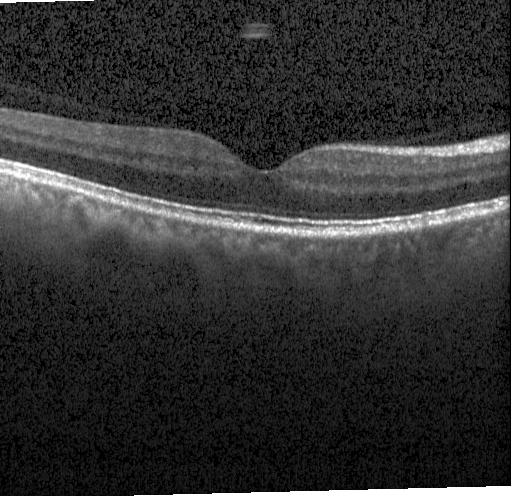 Optical coherence tomography scan. Diagnosis: no evidence of choroidal neovascularization, diabetic macular edema, or drusen.